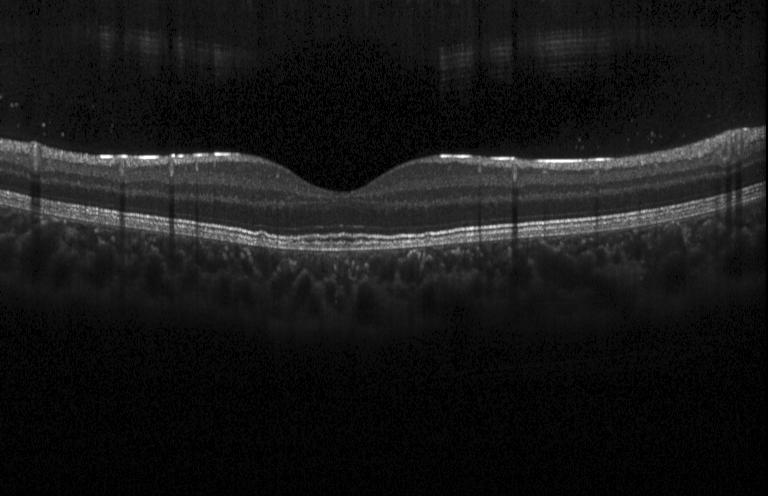 Retinal OCT B-scan — Assessment: no CNV, DME, or drusen.